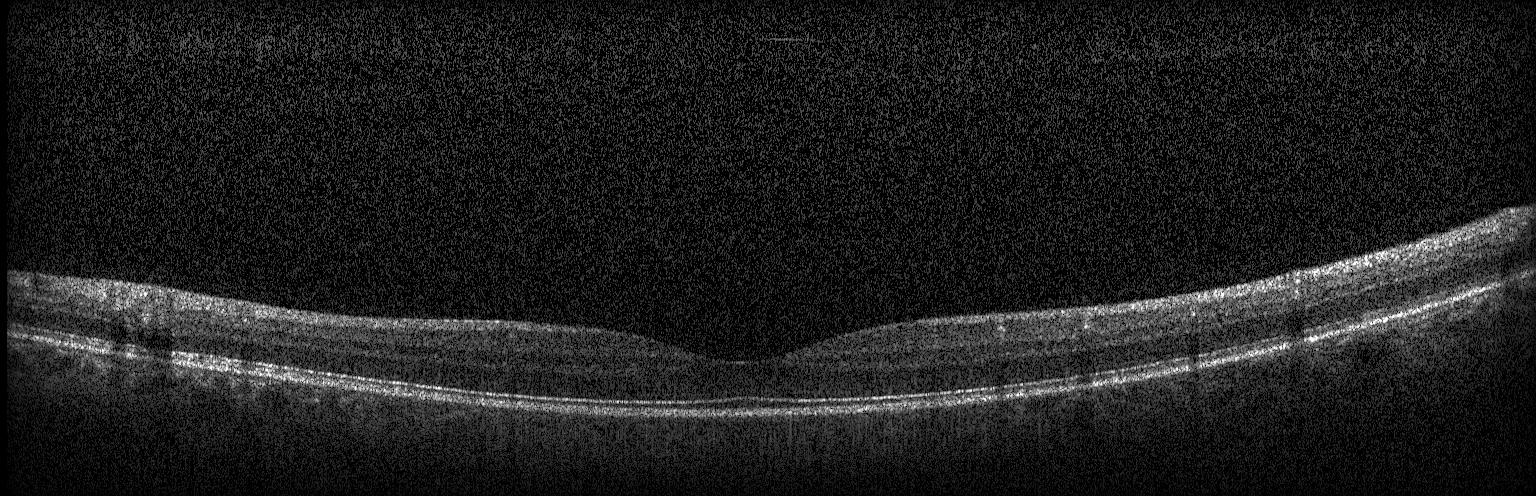
Heidelberg Spectralis OCT system; macular scan; optical coherence tomography scan; SD-OCT
Finding: neither choroidal neovascularization, diabetic macular edema, nor drusen.